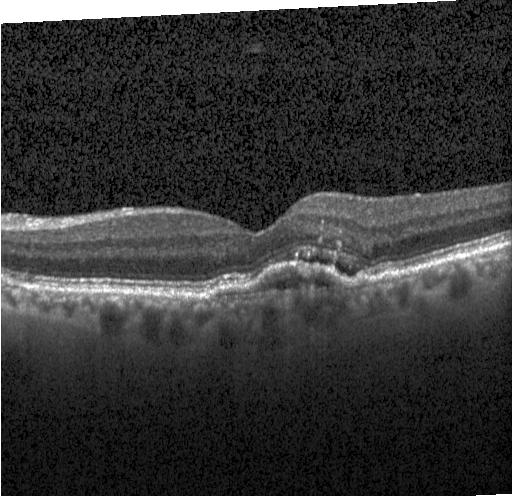 OCT B-scan. Finding: choroidal neovascularization (CNV).